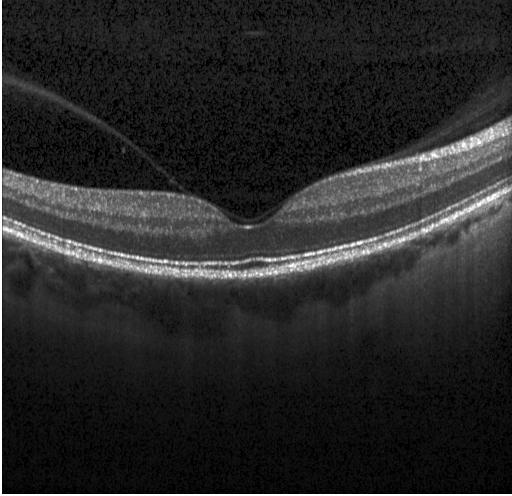 Diagnosis: no choroidal neovascularization, diabetic macular edema, or drusen.